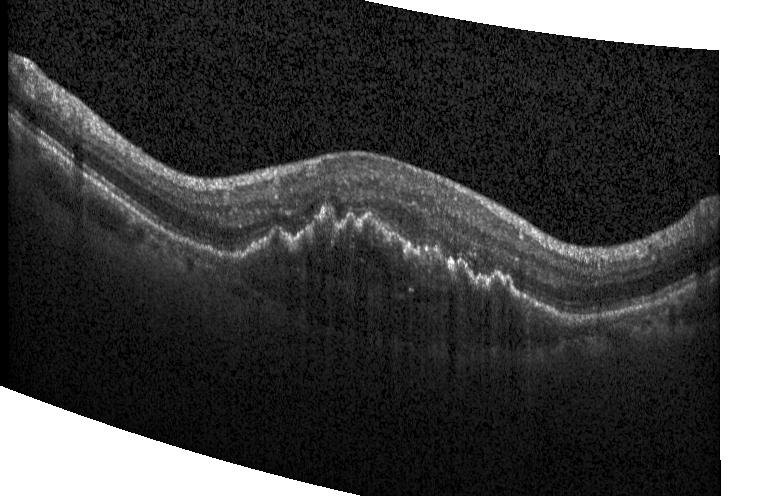
Retinal OCT B-scan; spectral-domain optical coherence tomography; instrument: Heidelberg Spectralis
Diagnosis: a choroidal neovascular membrane.